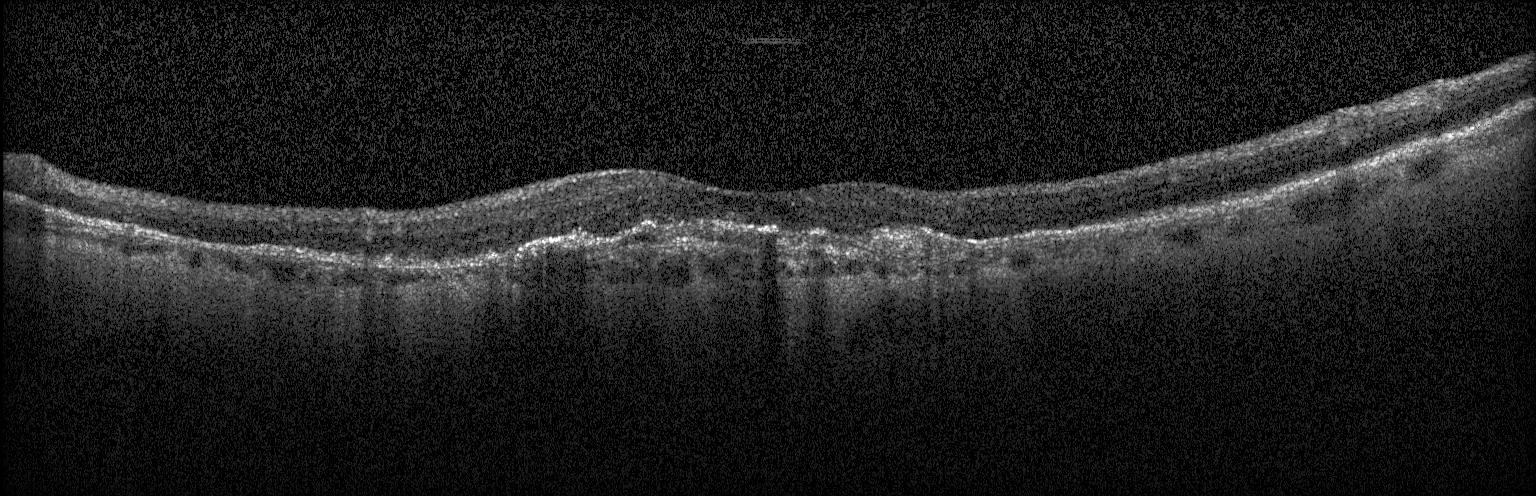 Retinal OCT cross-section · SD-OCT · acquired on a Heidelberg Spectralis.
Finding: a choroidal neovascular membrane.